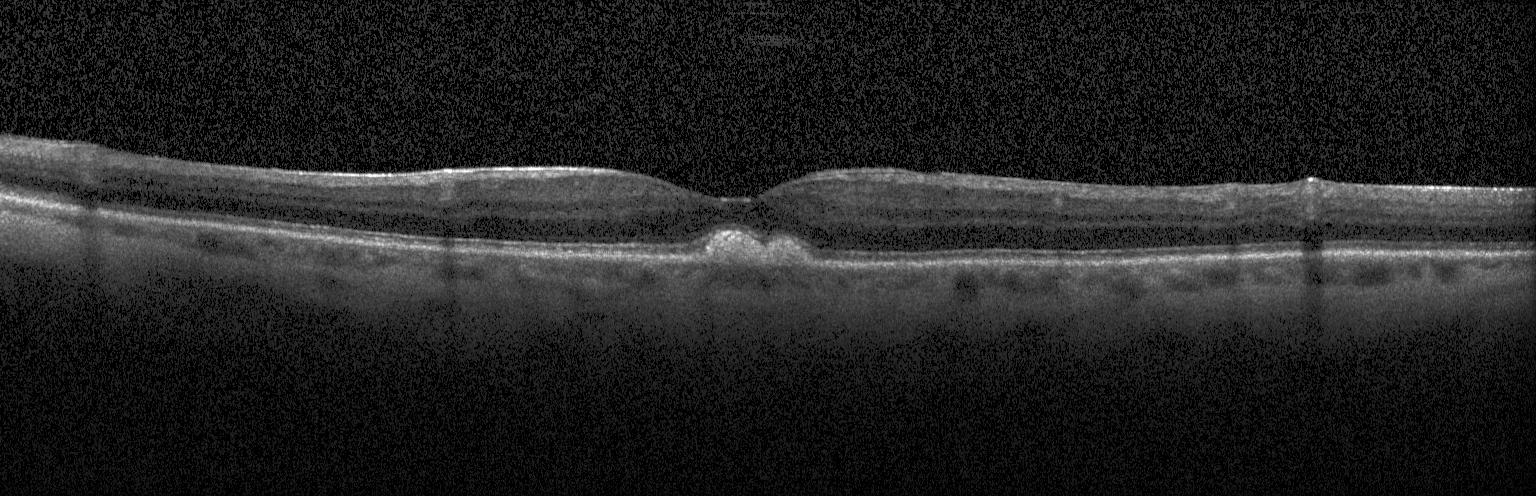

SD-OCT; through the macula; optical coherence tomography scan; Heidelberg Spectralis
Drusen.